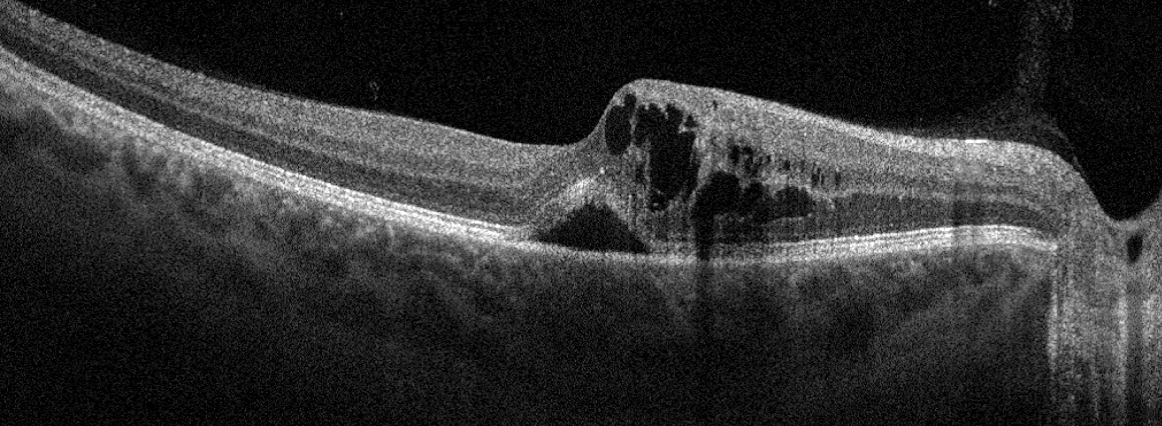

Through the macula; optical coherence tomography scan; oculus dexter.
Dx: RVO.